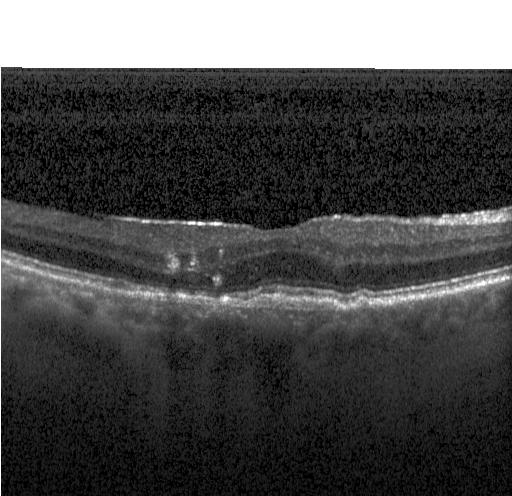

Retinal OCT cross-section showing CNV.